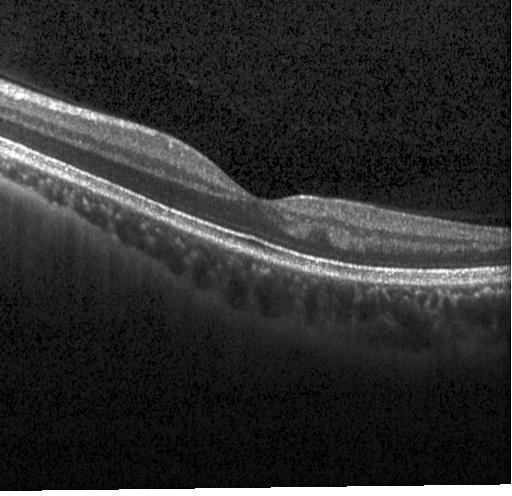
Spectral-domain optical coherence tomography · optical coherence tomography scan.
Impression: no choroidal neovascularization, diabetic macular edema, or drusen.